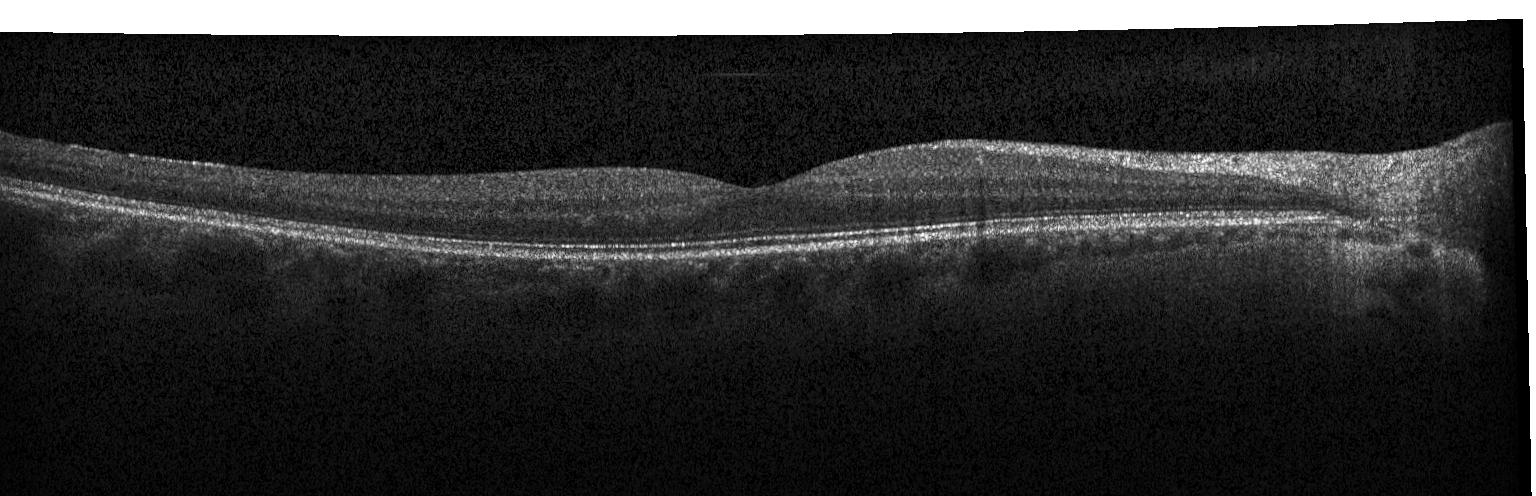

OCT B-scan showing no choroidal neovascularization, diabetic macular edema, or drusen.